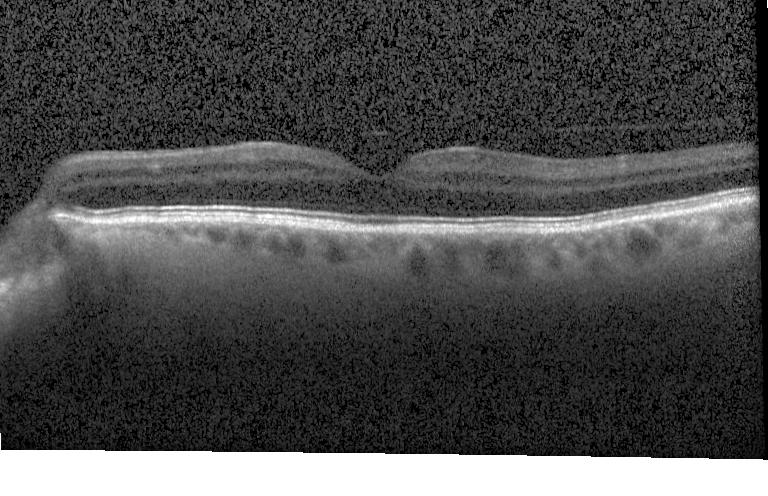 OCT B-scan showing no CNV, no DME, and no drusen.